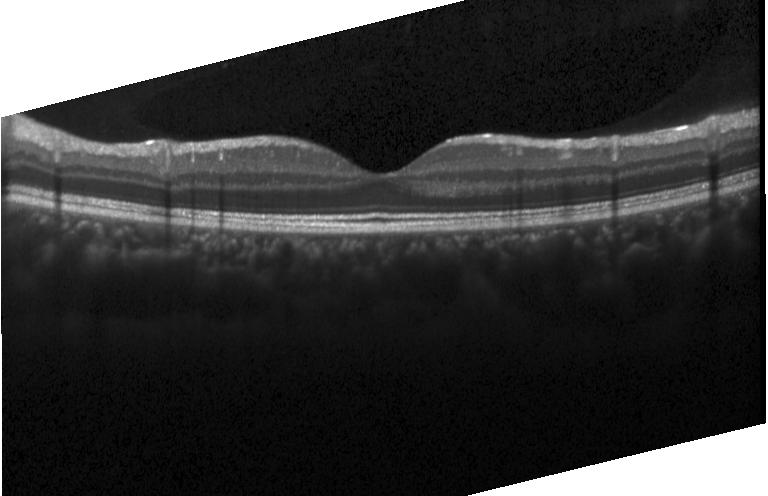
Optical coherence tomography B-scan, horizontal scan through the fovea, instrument: Heidelberg Spectralis, spectral-domain OCT. Impression: no CNV, no DME, and no drusen.